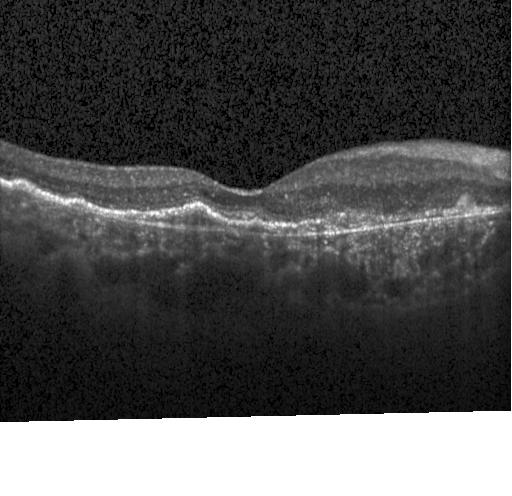
Finding: choroidal neovascularization.